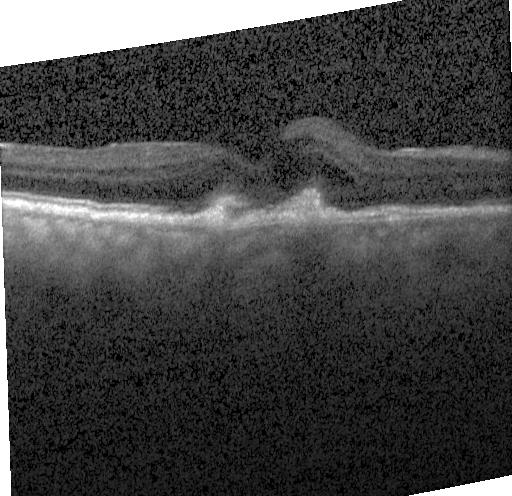

Retinal OCT B-scan; instrument: Heidelberg Spectralis; horizontal scan through the fovea. Choroidal neovascularization.